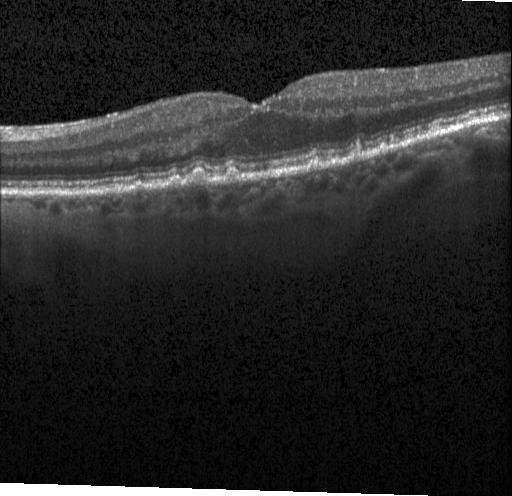
Macular OCT: sub-RPE drusenoid deposits.